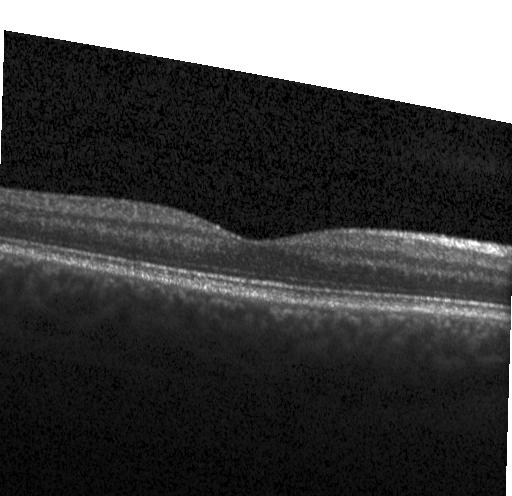

Optical coherence tomography B-scan · spectral-domain optical coherence tomography.
No evidence of CNV, DME, or drusen.